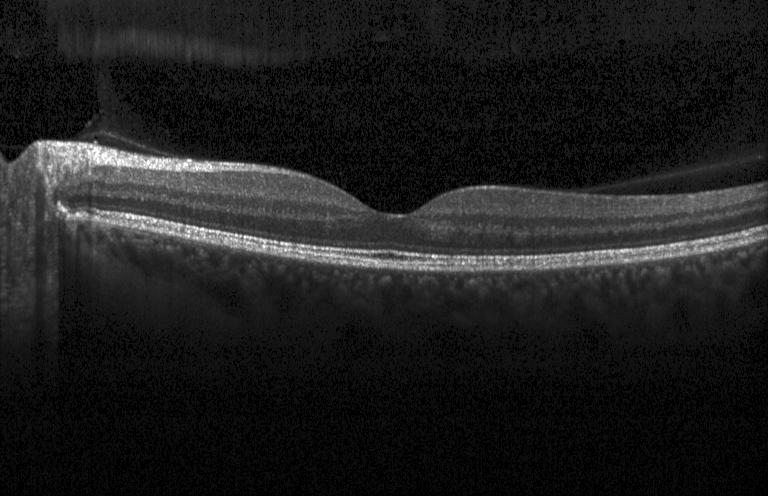

OCT line scan. Spectral-domain optical coherence tomography. Through the macula — Dx: no evidence of CNV, DME, or drusen.